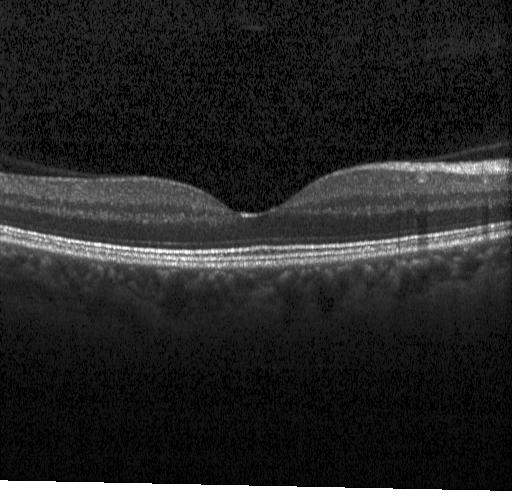 Optical coherence tomography scan
Finding: no choroidal neovascularization, no diabetic macular edema, and no drusen.